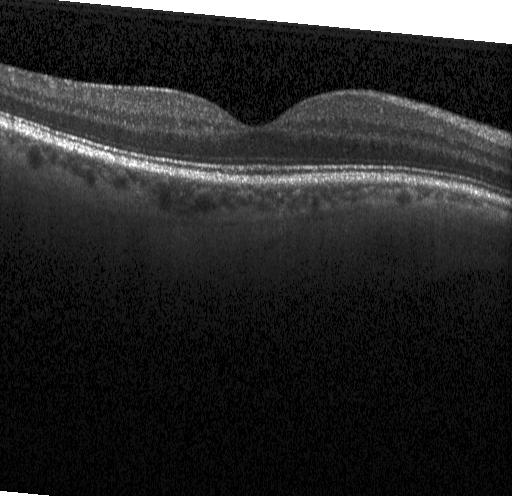

Heidelberg Spectralis; OCT line scan; fovea-centered; SD-OCT. Macular OCT: no evidence of CNV, DME, or drusen.